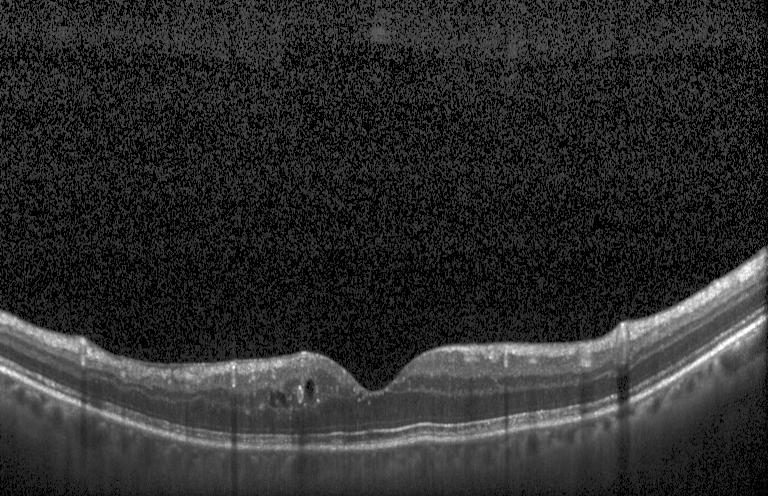 Optical coherence tomography scan
Diabetic macular edema (DME).